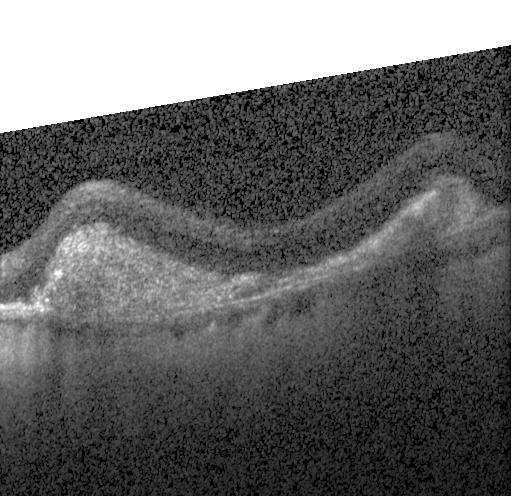
Instrument: Heidelberg Spectralis, optical coherence tomography scan — Finding: a choroidal neovascular membrane.